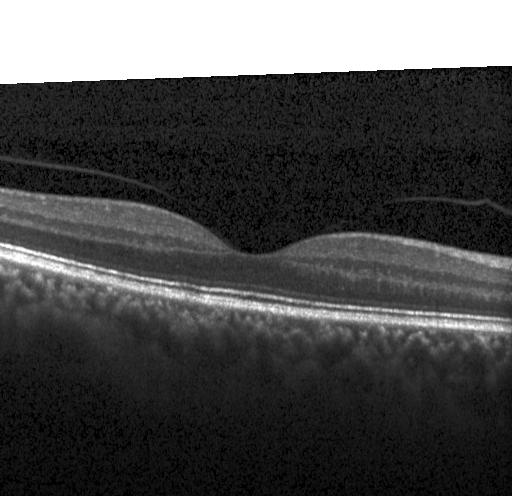

Retinal OCT B-scan; instrument: Heidelberg Spectralis; spectral-domain optical coherence tomography. Macular OCT: no choroidal neovascularization, diabetic macular edema, or drusen.